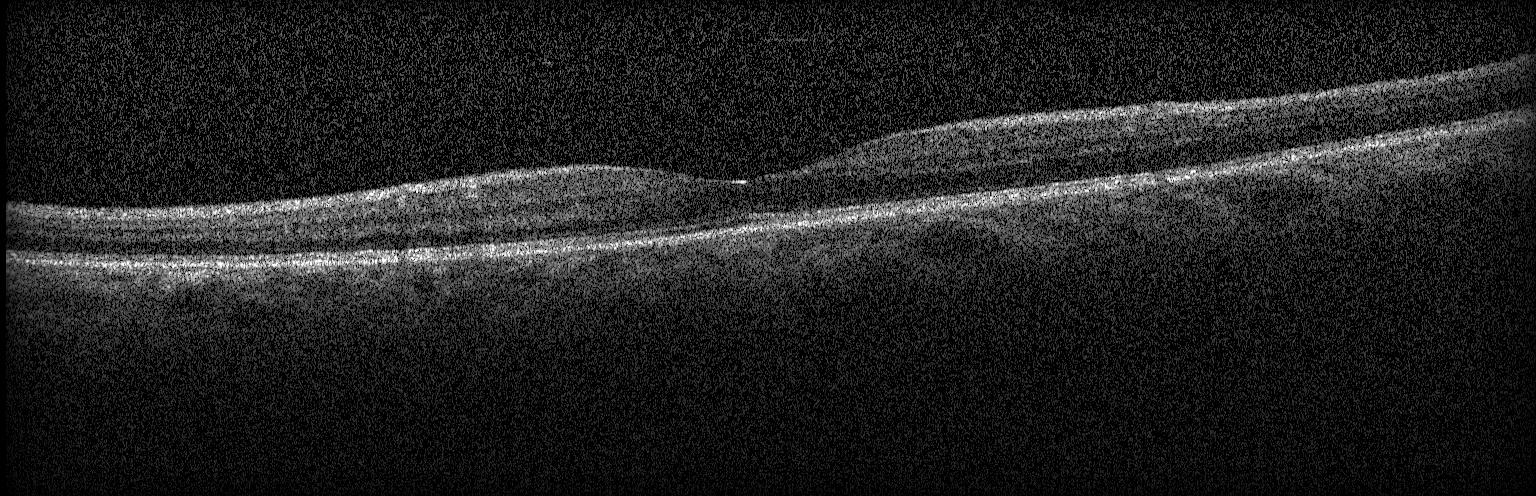

Retinal OCT B-scan · Heidelberg Spectralis · SD-OCT — Macular OCT: no choroidal neovascularization, no diabetic macular edema, and no drusen.